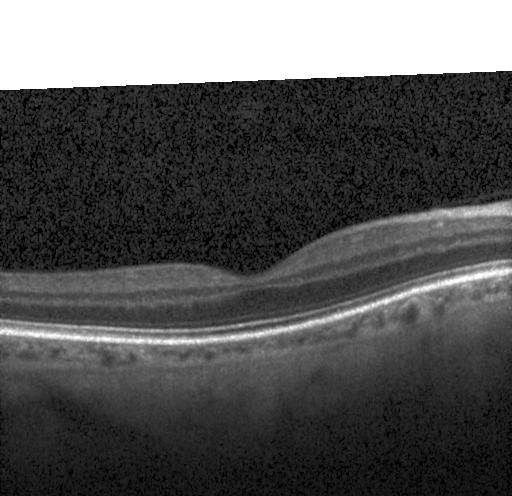

Macular OCT: no choroidal neovascularization, diabetic macular edema, or drusen.